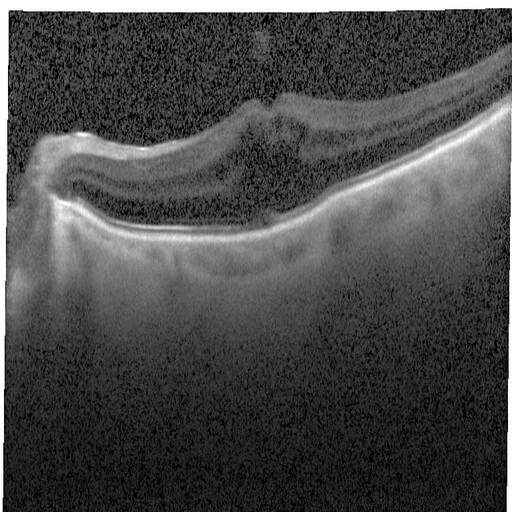
Horizontal scan through the fovea. Optical coherence tomography B-scan. Heidelberg Spectralis — Finding: diabetic macular edema (DME).